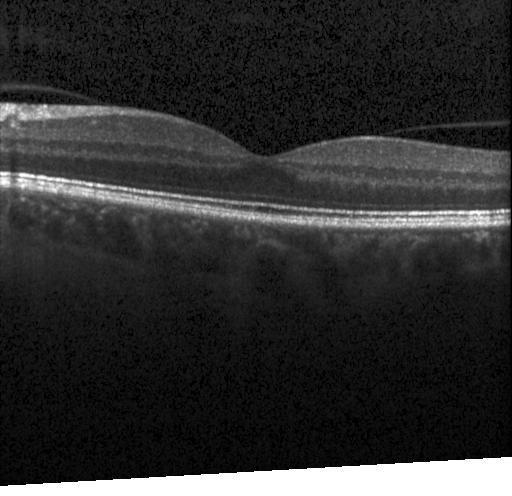
Spectral-domain OCT. Instrument: Heidelberg Spectralis. OCT B-scan — Finding: no choroidal neovascularization, no diabetic macular edema, and no drusen.